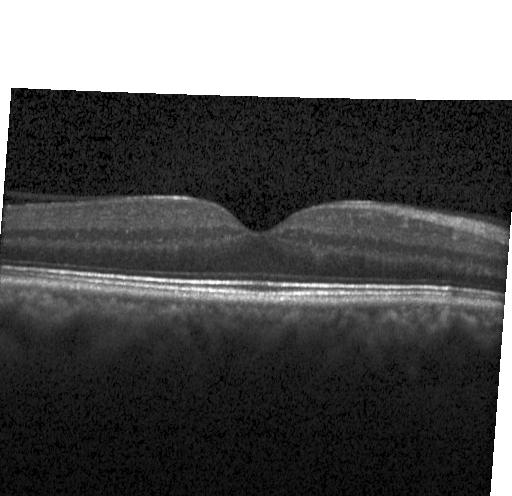
OCT B-scan showing no choroidal neovascularization, diabetic macular edema, or drusen.